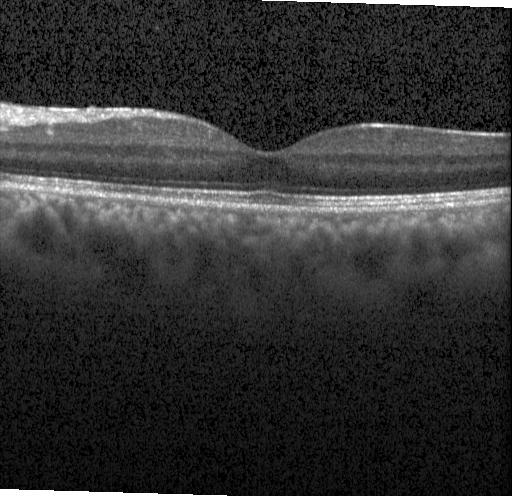
OCT line scan; spectral-domain optical coherence tomography
Finding: no evidence of choroidal neovascularization, diabetic macular edema, or drusen.